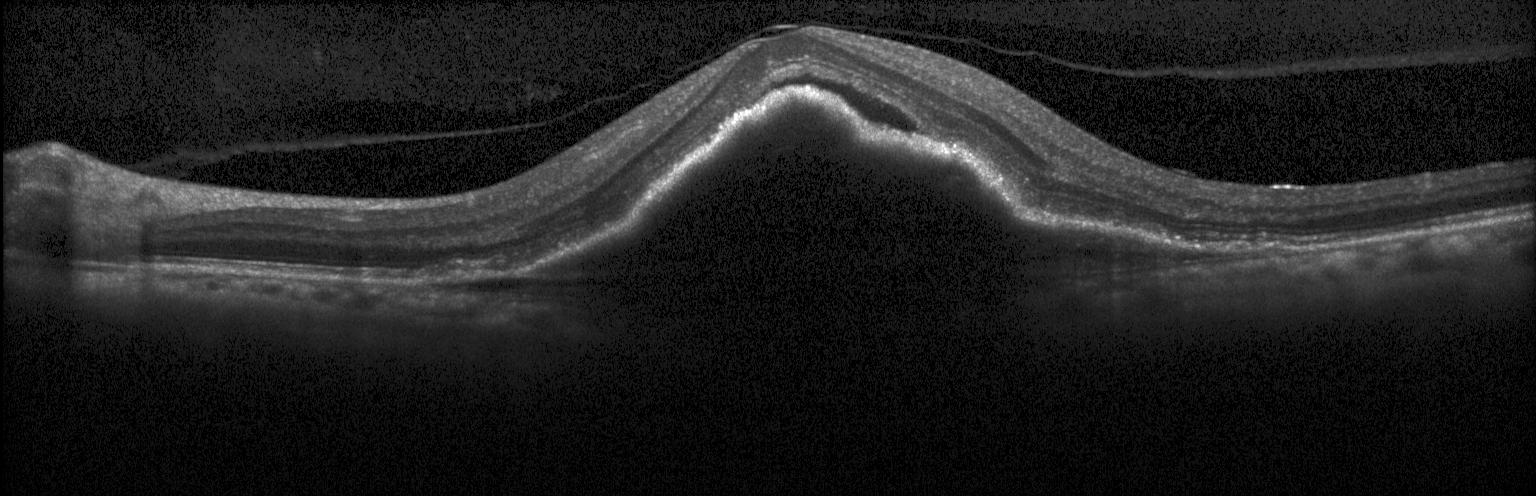

OCT B-scan showing a choroidal neovascular membrane.